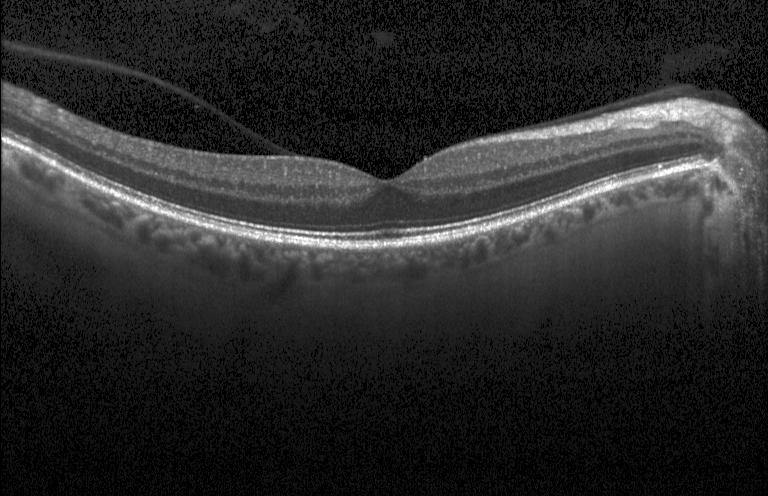 OCT B-scan · Heidelberg Spectralis OCT system. This B-scan demonstrates neither choroidal neovascularization, diabetic macular edema, nor drusen.